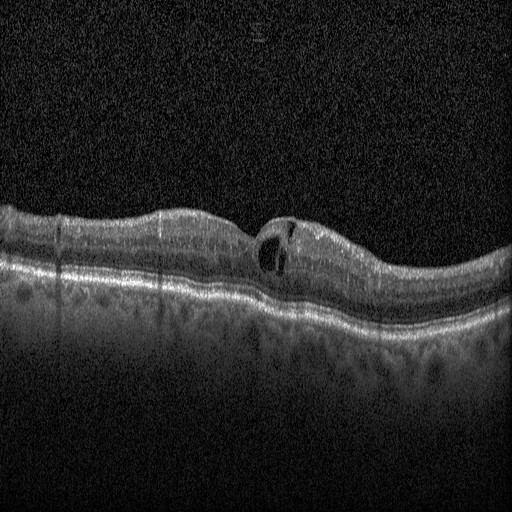

Instrument: Heidelberg Spectralis · retinal OCT B-scan · spectral-domain OCT · centered on the fovea
Diabetic macular edema (DME).